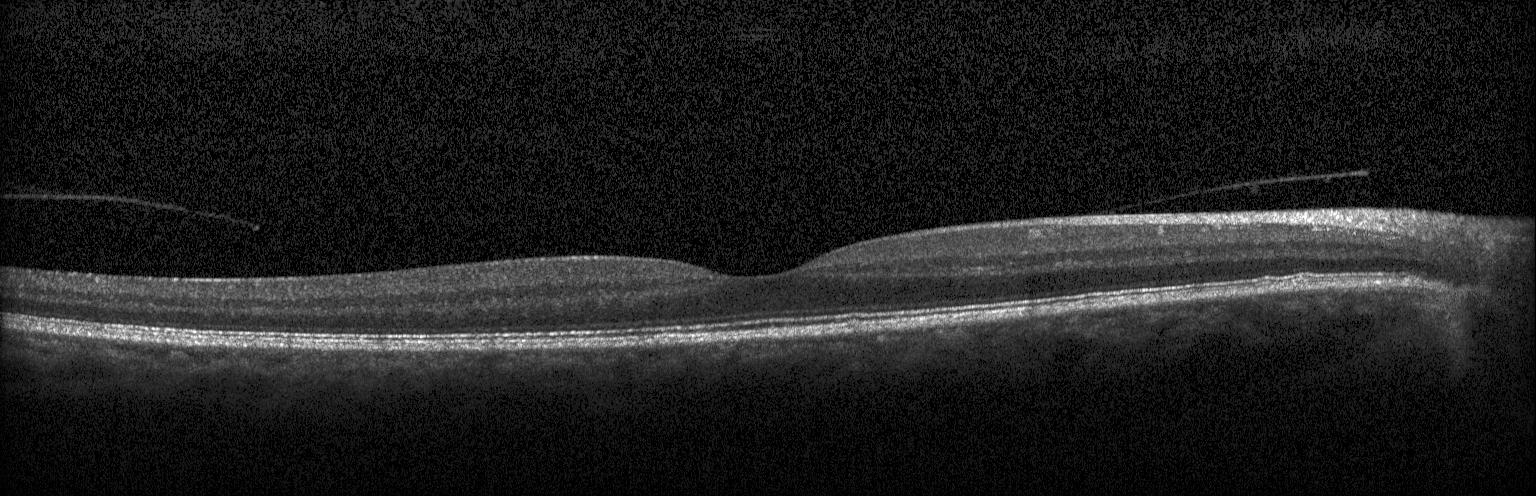
Impression: no choroidal neovascularization, no diabetic macular edema, and no drusen.